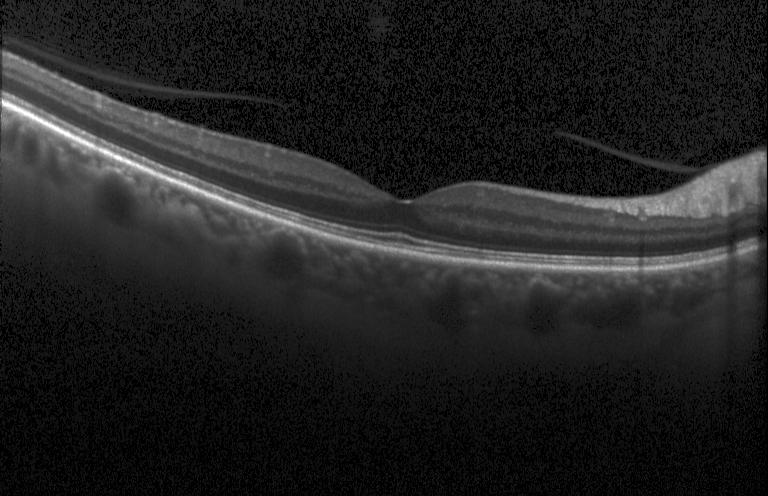

Retinal OCT B-scan. Impression: neither choroidal neovascularization, diabetic macular edema, nor drusen.